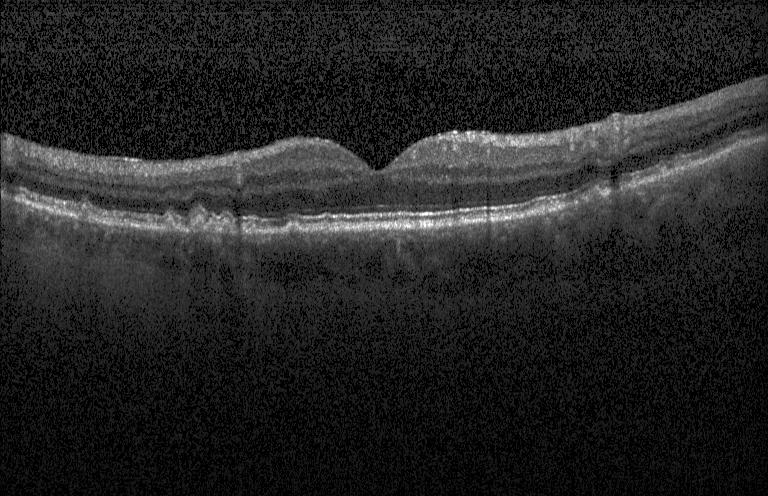

OCT B-scan, horizontal scan through the fovea, SD-OCT
Finding: sub-RPE drusenoid deposits.